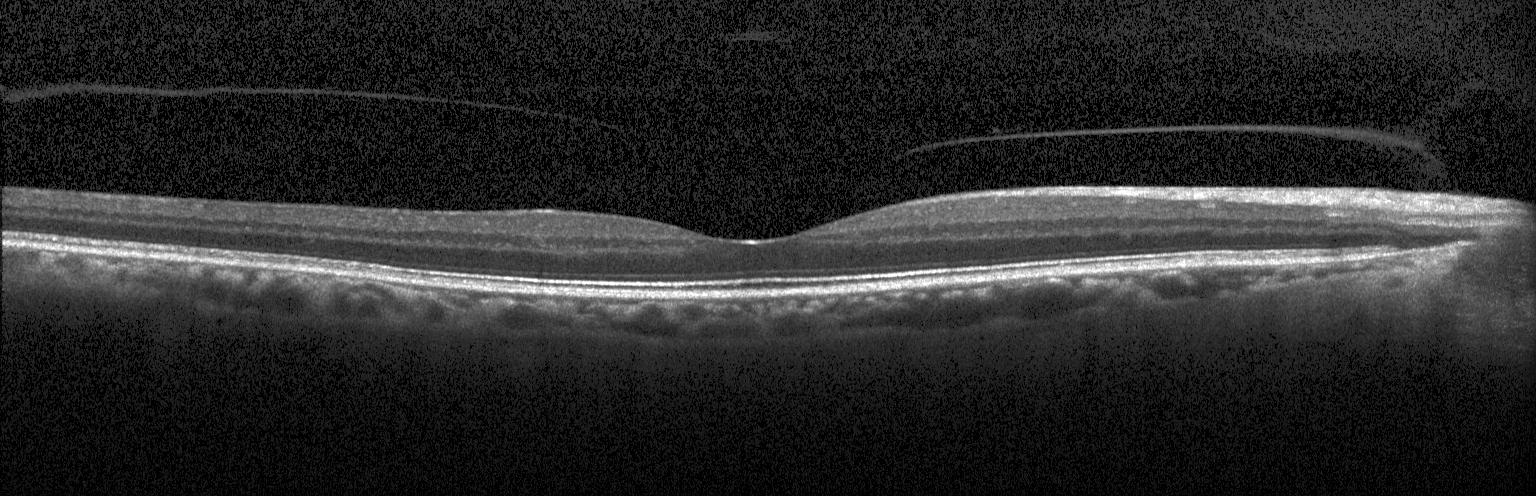 Impression: no evidence of CNV, DME, or drusen.